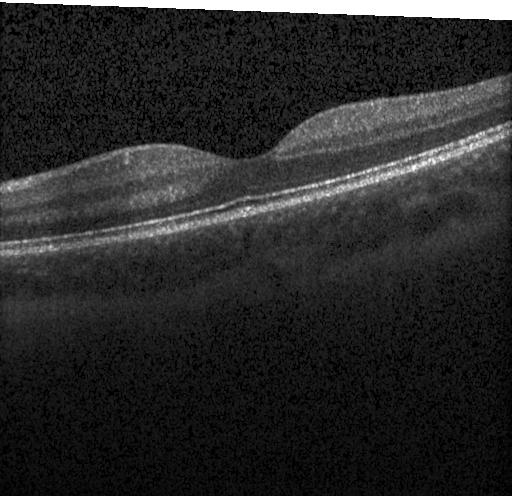

Finding: no evidence of CNV, DME, or drusen.